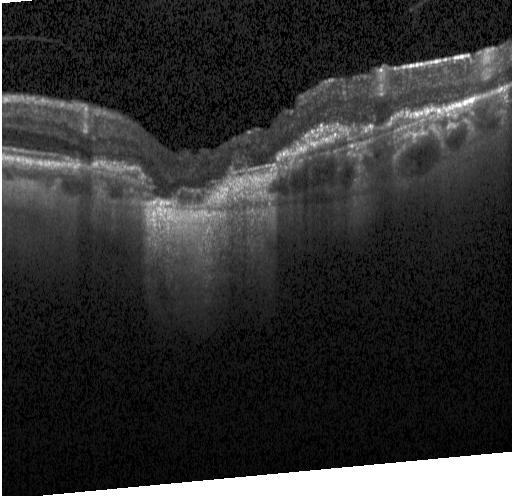
SD-OCT. Heidelberg Spectralis. Fovea-centered. Retinal OCT B-scan.
Assessment: choroidal neovascularization (CNV).